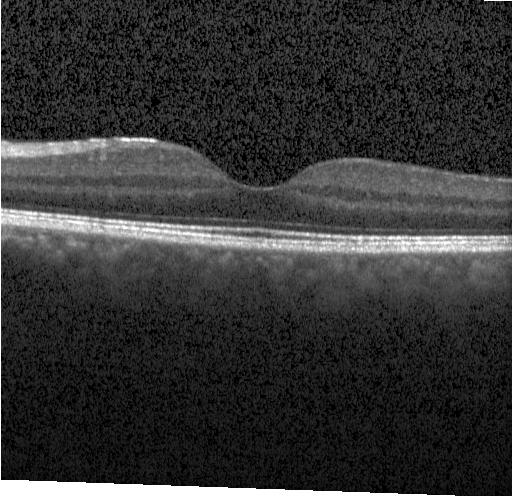

OCT line scan, spectral-domain OCT
Impression: no evidence of CNV, DME, or drusen.